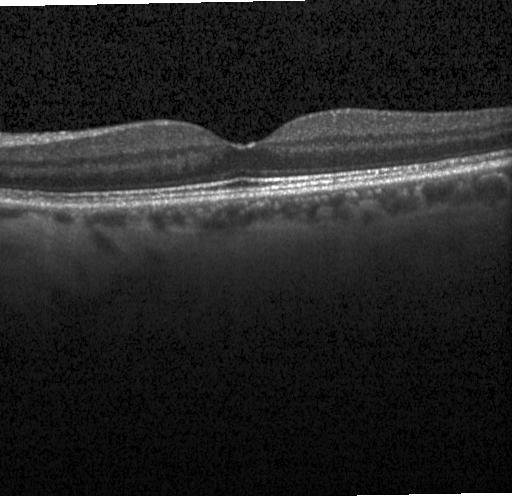 Diagnosis: no choroidal neovascularization, diabetic macular edema, or drusen.